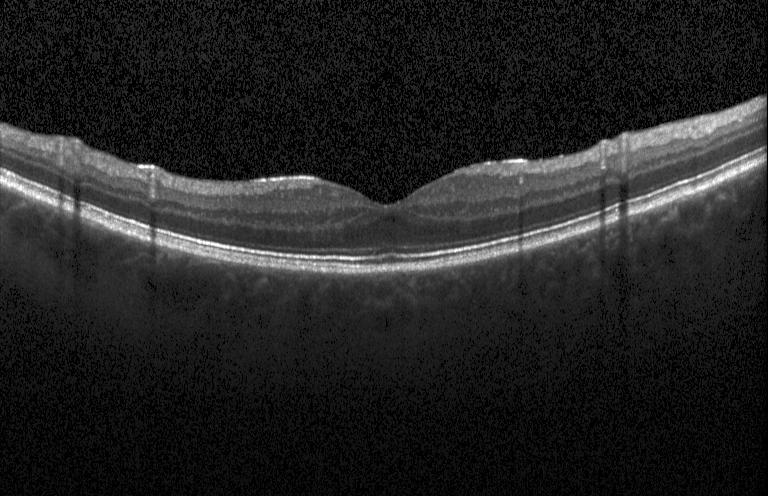
Fovea-centered. Heidelberg Spectralis OCT system. SD-OCT. Retinal OCT B-scan — Assessment: neither choroidal neovascularization, diabetic macular edema, nor drusen.